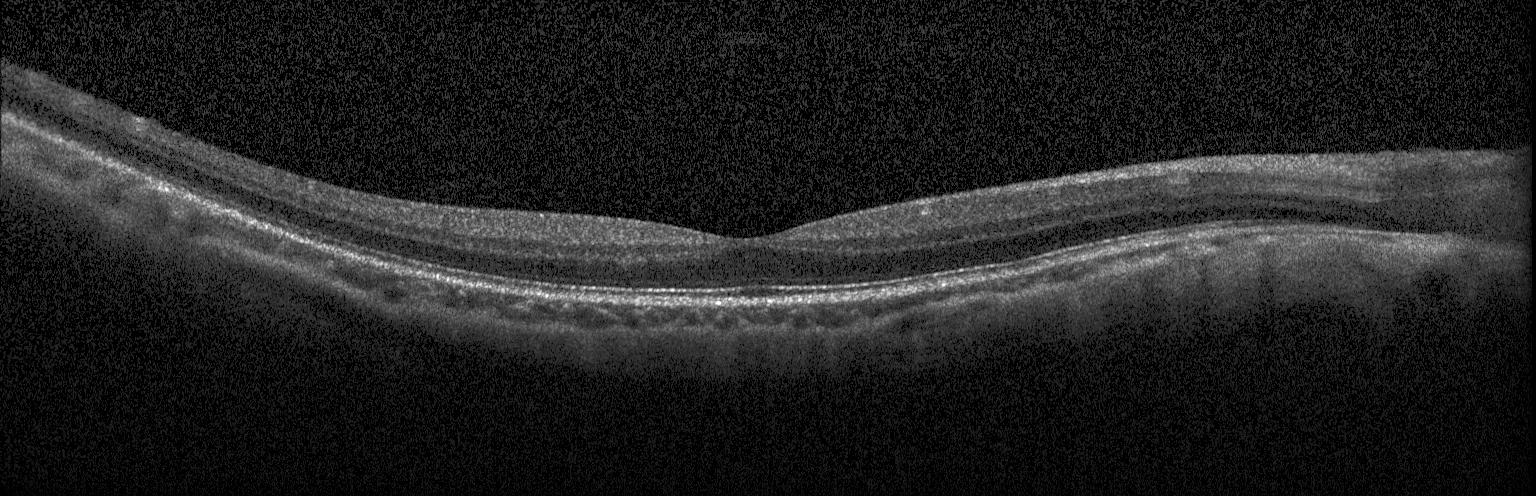
Finding: no evidence of choroidal neovascularization, diabetic macular edema, or drusen.